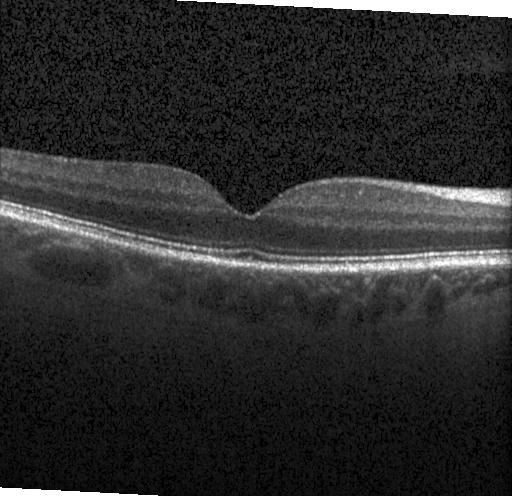 Retinal OCT cross-section showing no choroidal neovascularization, no diabetic macular edema, and no drusen.